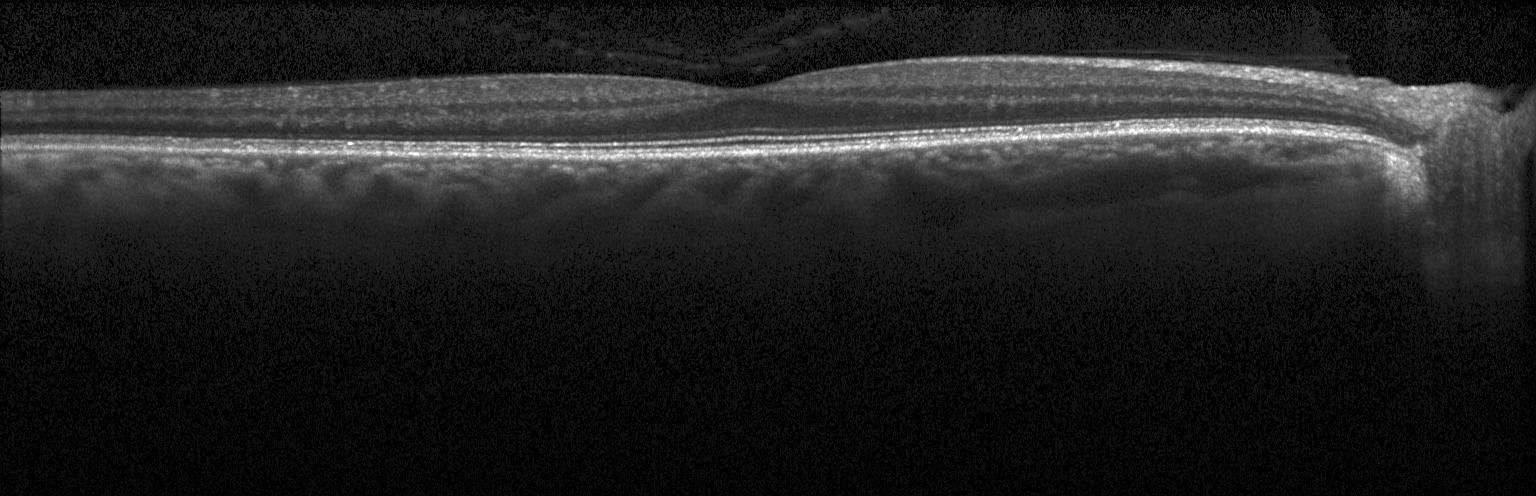

Instrument: Heidelberg Spectralis. OCT B-scan. Impression: no choroidal neovascularization, diabetic macular edema, or drusen.